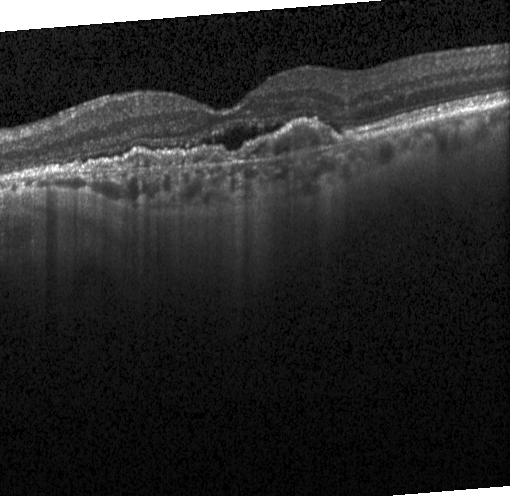
Impression: a choroidal neovascular membrane.